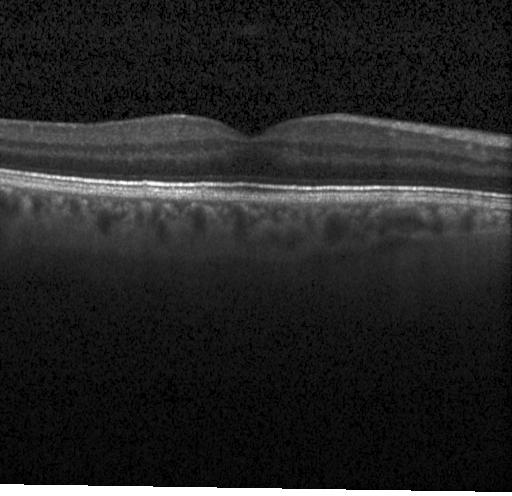 Horizontal scan through the fovea, optical coherence tomography scan.
Finding: no evidence of choroidal neovascularization, diabetic macular edema, or drusen.